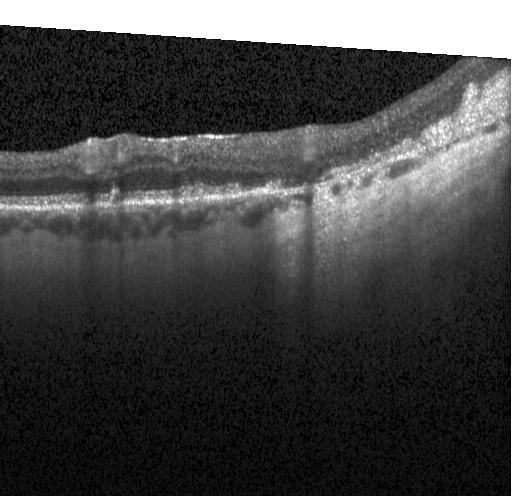

Retinal OCT B-scan — Diagnosis: choroidal neovascularization.